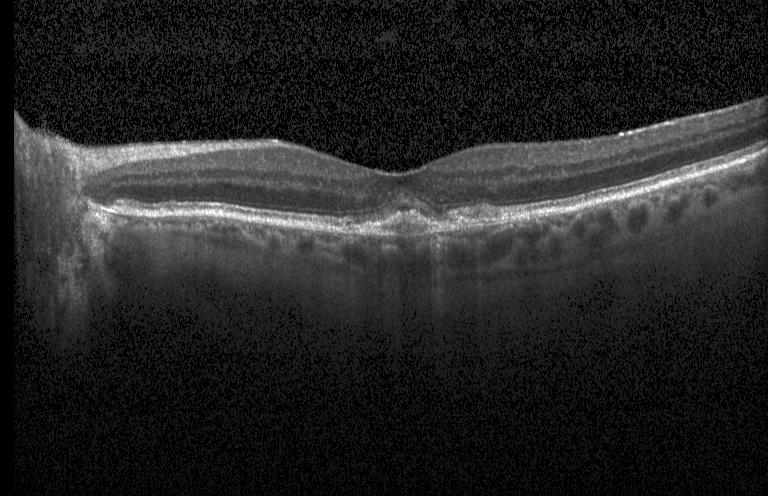

Spectral-domain optical coherence tomography; through the macula; instrument: Heidelberg Spectralis; optical coherence tomography B-scan
OCT finding: a choroidal neovascular membrane.